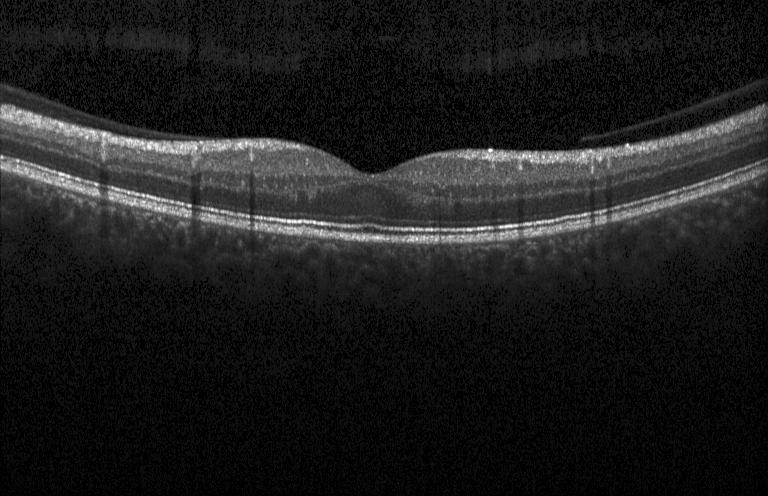 This B-scan demonstrates no choroidal neovascularization, no diabetic macular edema, and no drusen.